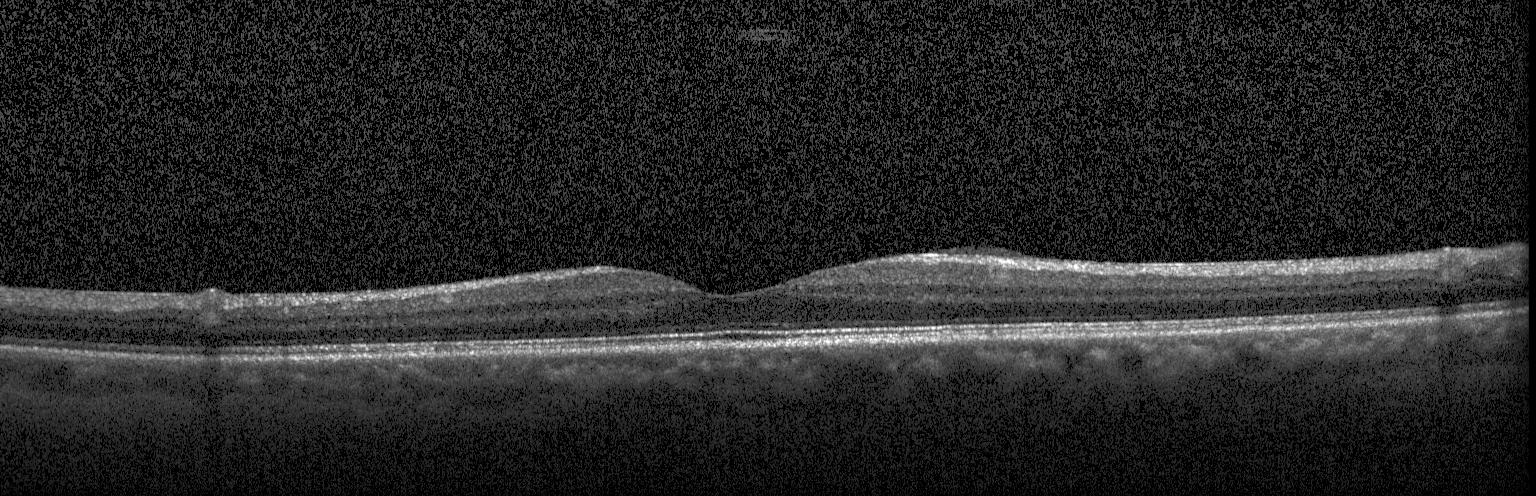 Diagnosis: no choroidal neovascularization, no diabetic macular edema, and no drusen.